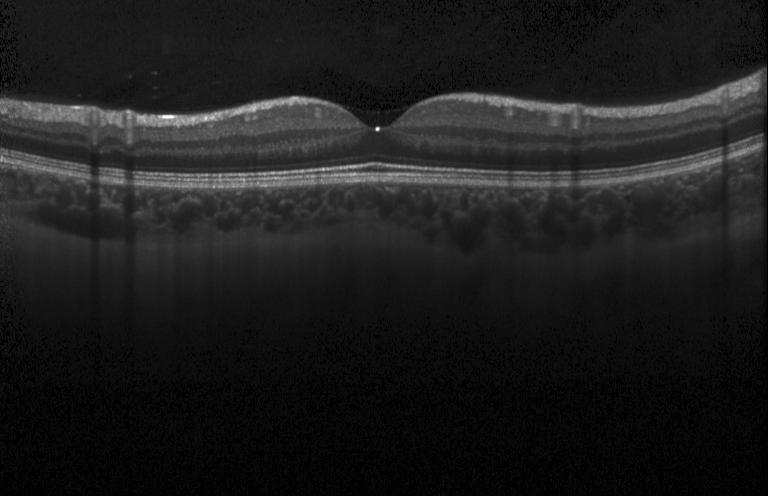 Diagnosis: no choroidal neovascularization, diabetic macular edema, or drusen.